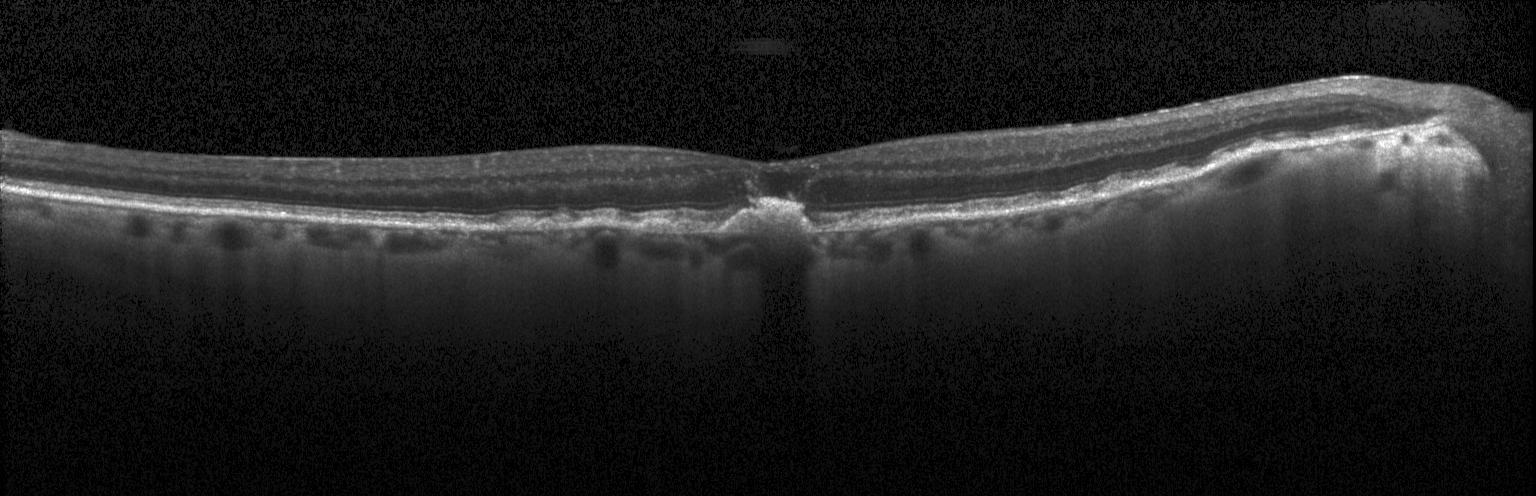
SD-OCT, optical coherence tomography B-scan, Heidelberg Spectralis, horizontal scan through the fovea. Finding: multiple drusen.